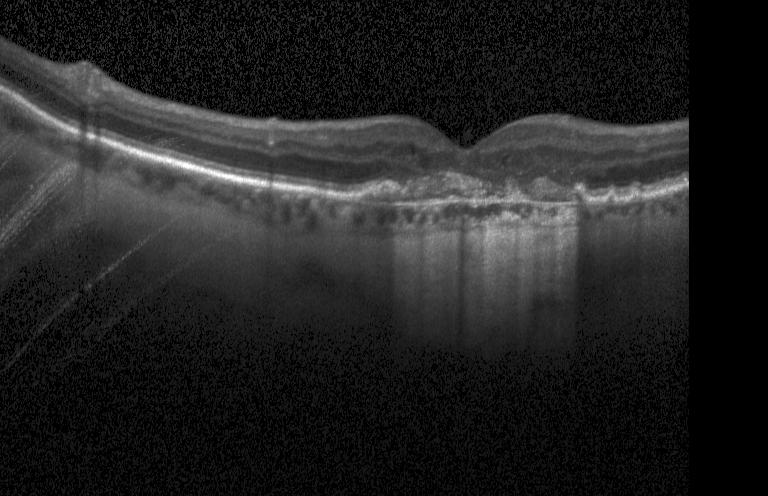

Macular scan · spectral-domain OCT · retinal OCT cross-section. Dx: CNV.